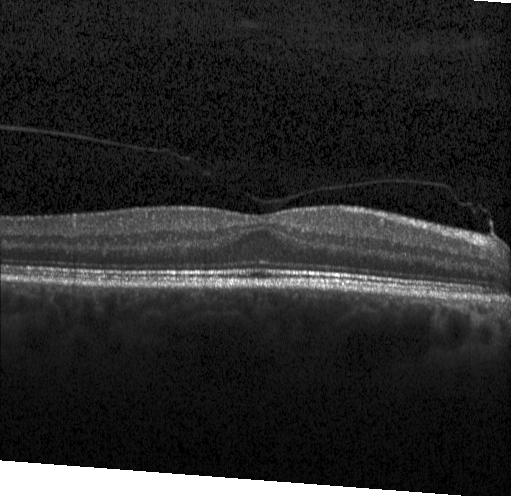

Diagnosis: no choroidal neovascularization, no diabetic macular edema, and no drusen.